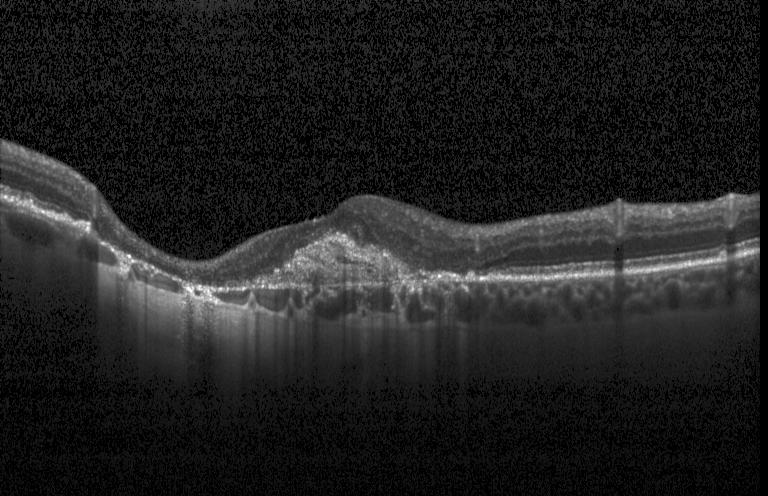

Diagnosis: choroidal neovascularization.